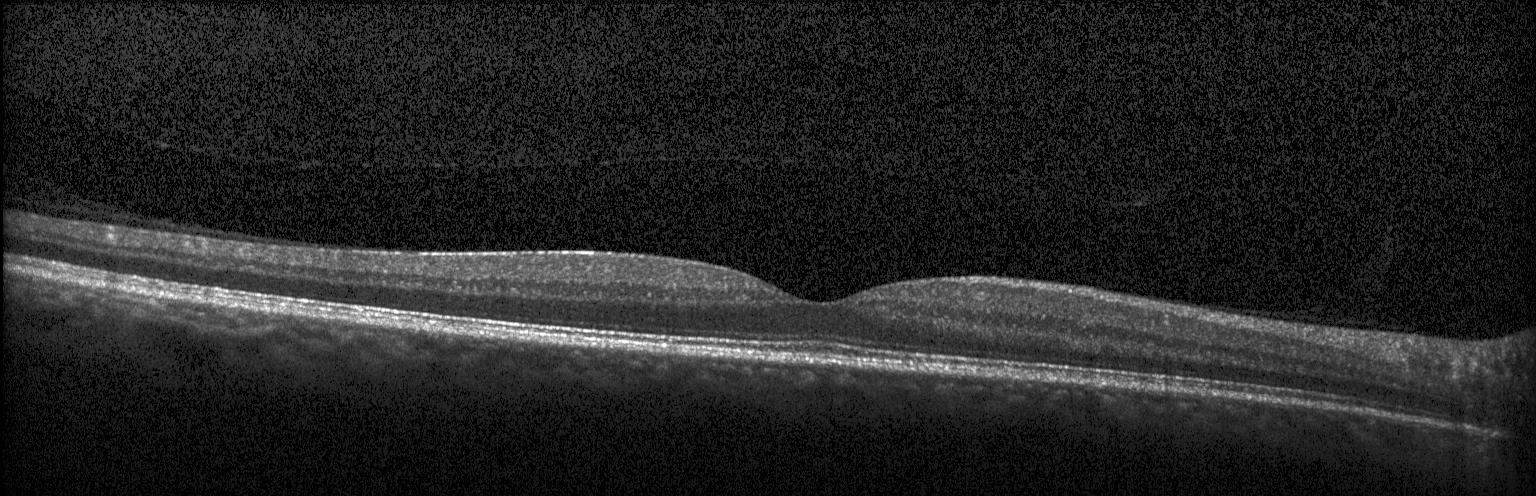

Retinal OCT cross-section — Assessment: no CNV, DME, or drusen.